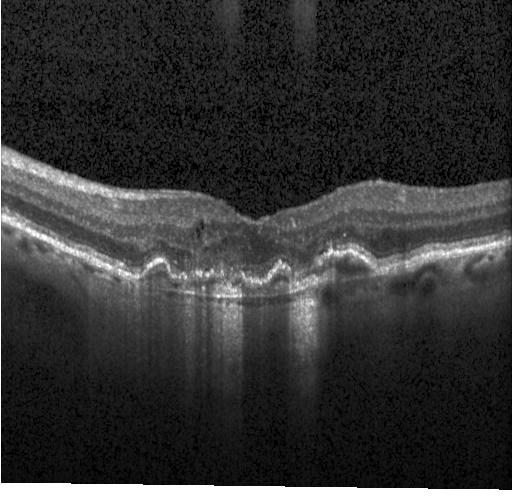 Macular OCT: choroidal neovascularization.